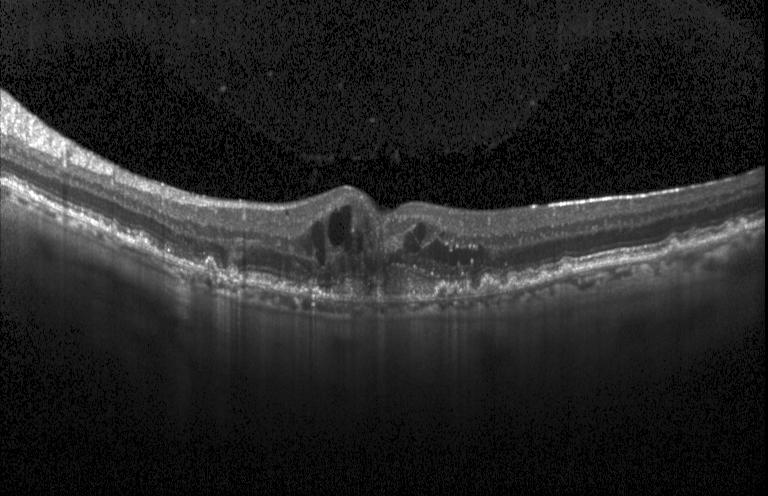

Macular scan, acquired on a Heidelberg Spectralis, spectral-domain OCT, optical coherence tomography B-scan
Dx: CNV.